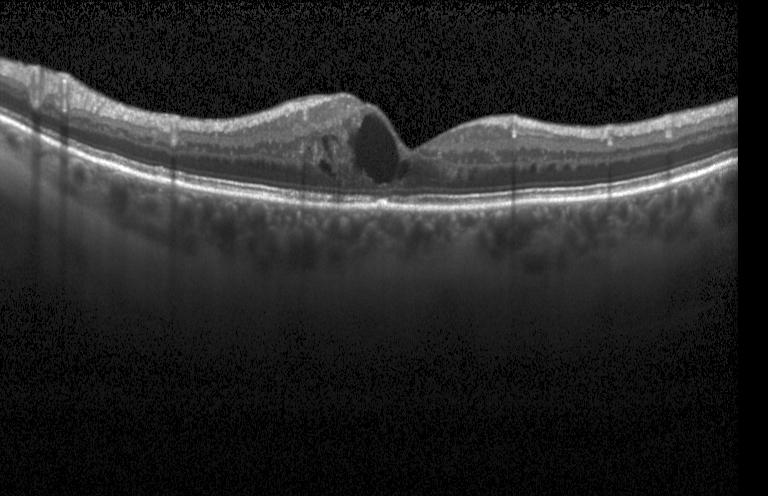 Diabetic macular edema.